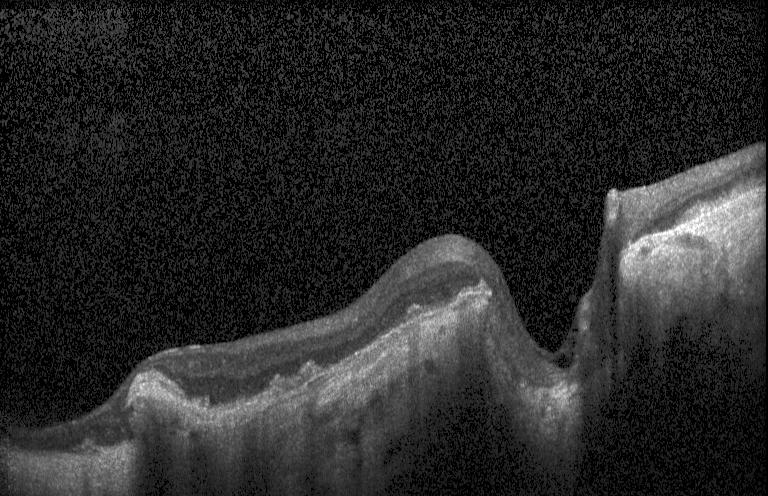
Impression: a choroidal neovascular membrane.